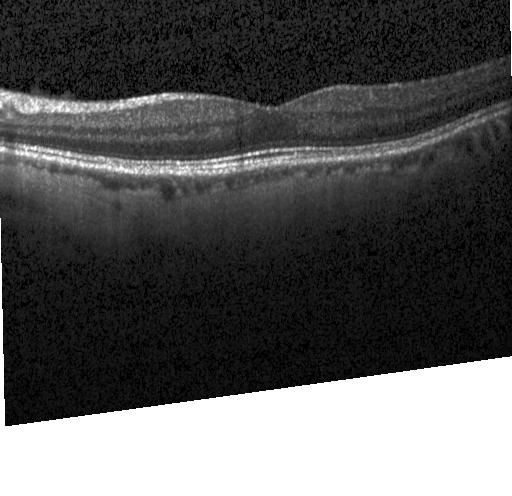
Assessment: no choroidal neovascularization, diabetic macular edema, or drusen.